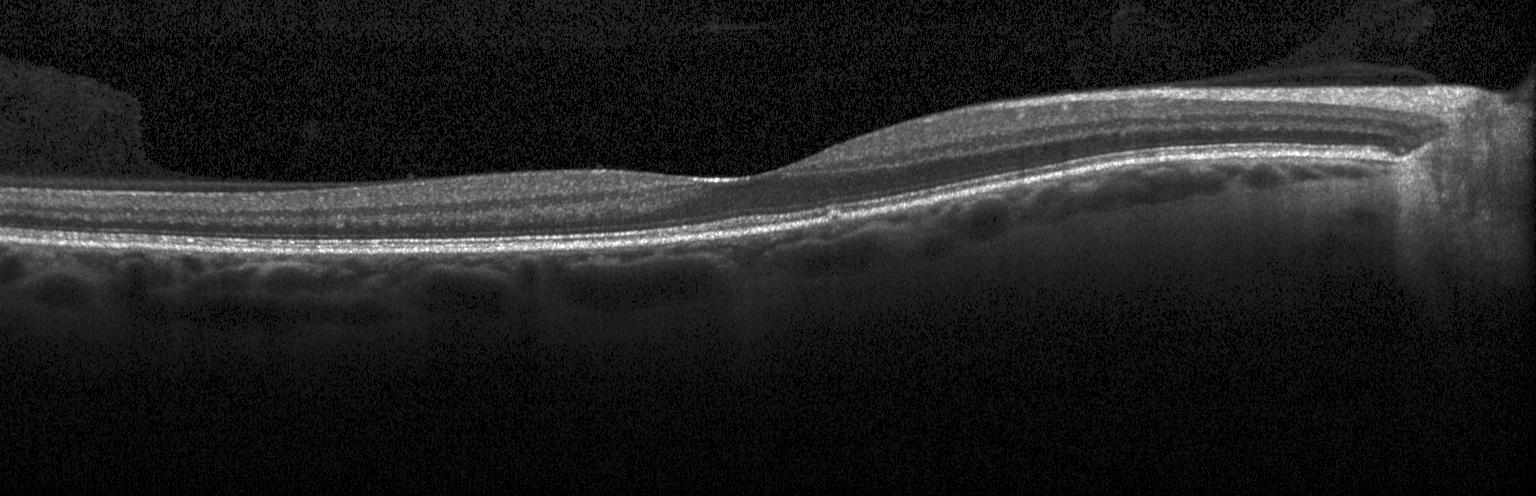
Spectral-domain OCT B-scan: no evidence of CNV, DME, or drusen.